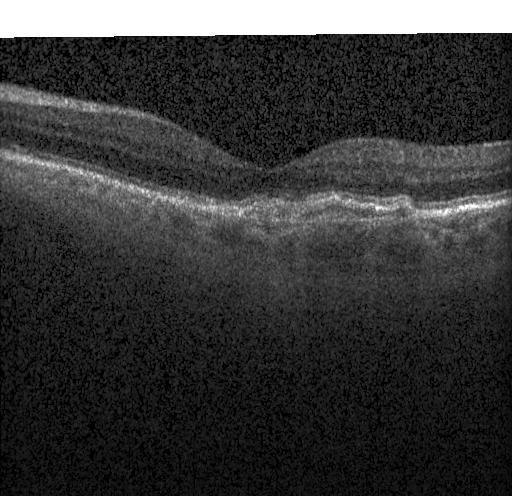

Dx: a choroidal neovascular membrane.